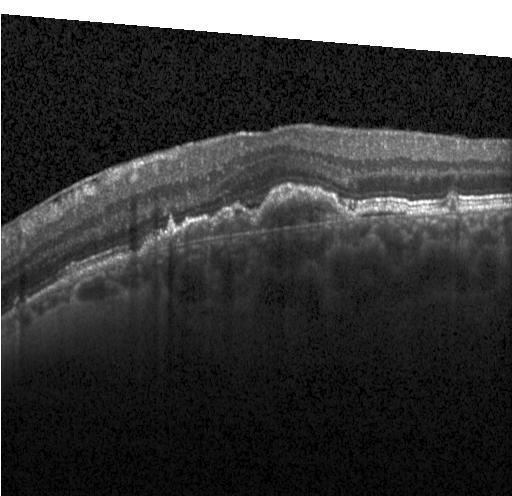 Diagnosis: CNV.